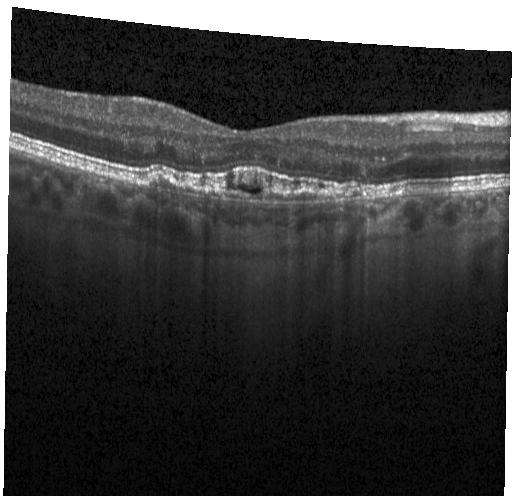 Finding: CNV.